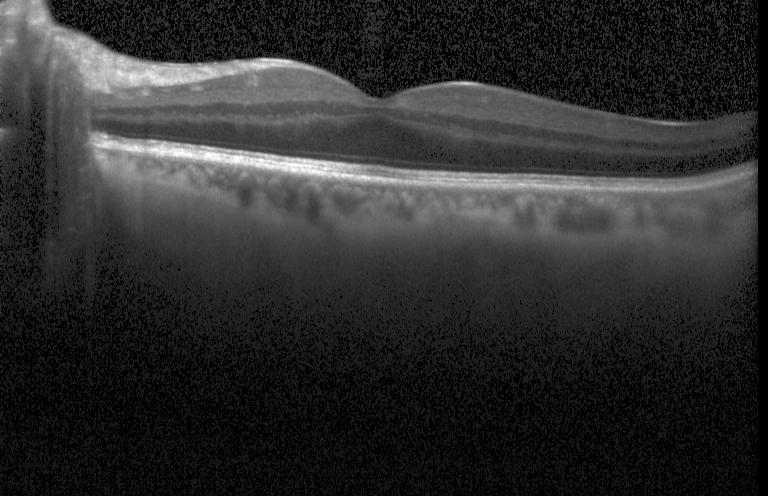 Spectral-domain optical coherence tomography; optical coherence tomography scan — Assessment: neither choroidal neovascularization, diabetic macular edema, nor drusen.